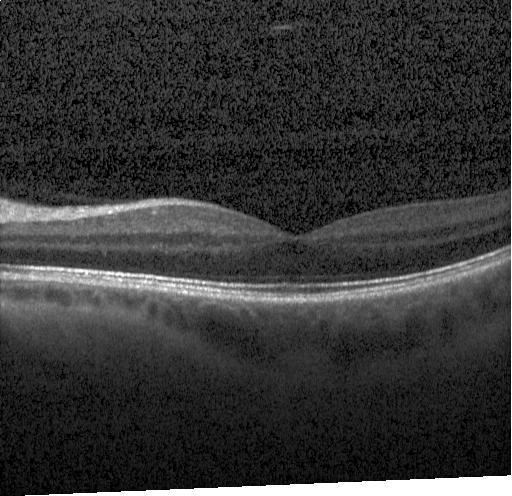 Horizontal scan through the fovea; optical coherence tomography scan — Diagnosis: no choroidal neovascularization, no diabetic macular edema, and no drusen.